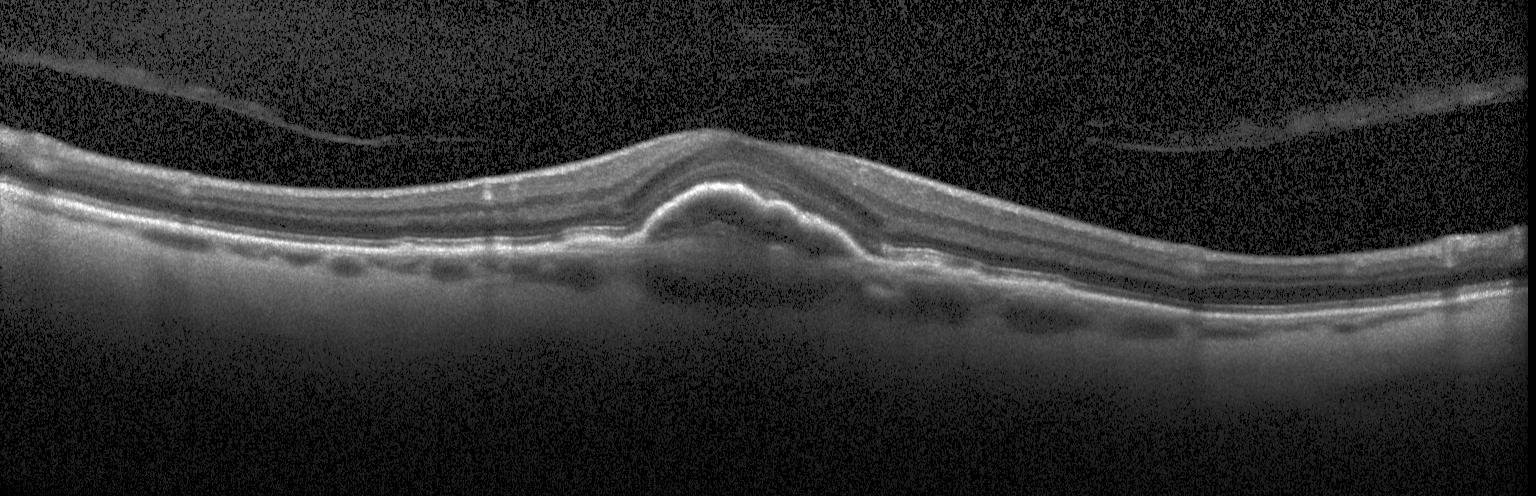
Diagnosis: a choroidal neovascular membrane.